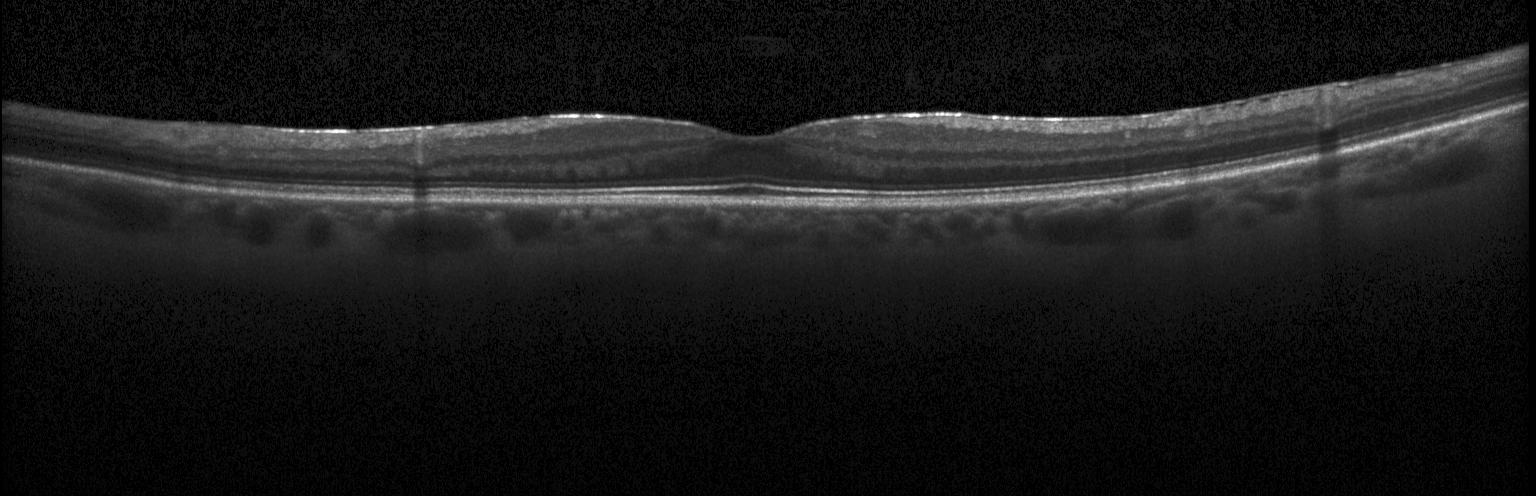 Macular OCT: no evidence of choroidal neovascularization, diabetic macular edema, or drusen.